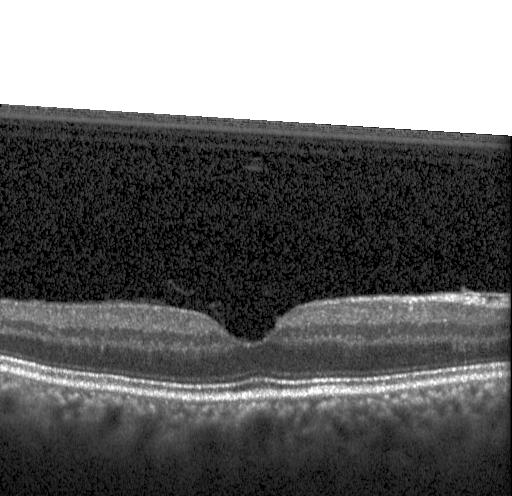 Acquired on a Heidelberg Spectralis · retinal OCT cross-section — Diagnosis: neither choroidal neovascularization, diabetic macular edema, nor drusen.